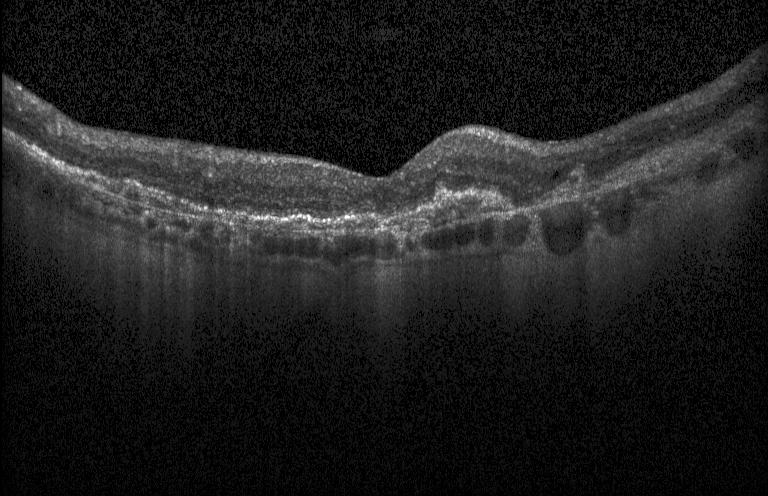

OCT line scan. Diagnosis: CNV.